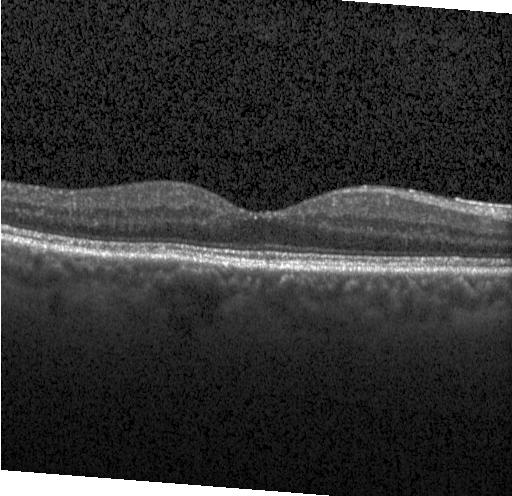
Spectral-domain optical coherence tomography. Instrument: Heidelberg Spectralis. Retinal OCT B-scan. Fovea-centered.
Finding: no choroidal neovascularization, no diabetic macular edema, and no drusen.